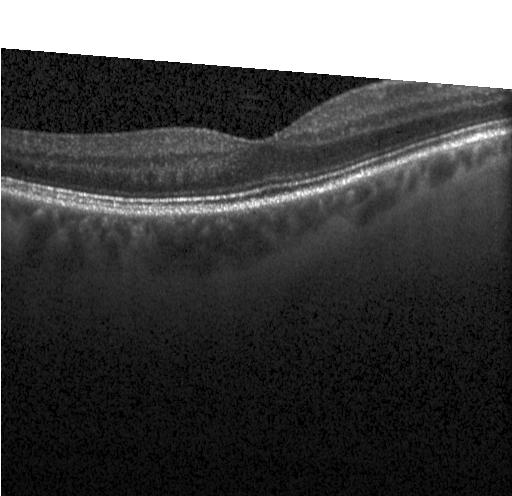 Retinal OCT B-scan
Impression: no choroidal neovascularization, diabetic macular edema, or drusen.